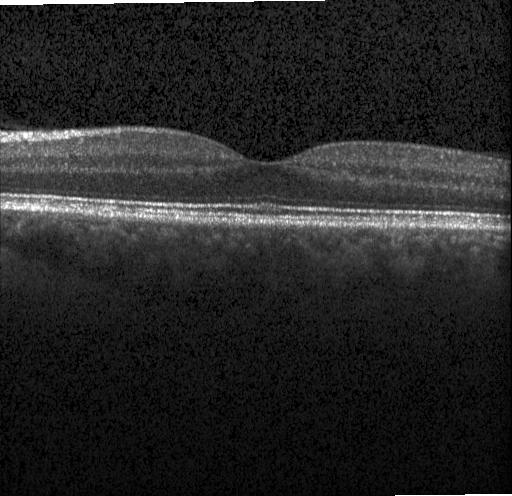 Finding: no choroidal neovascularization, diabetic macular edema, or drusen.